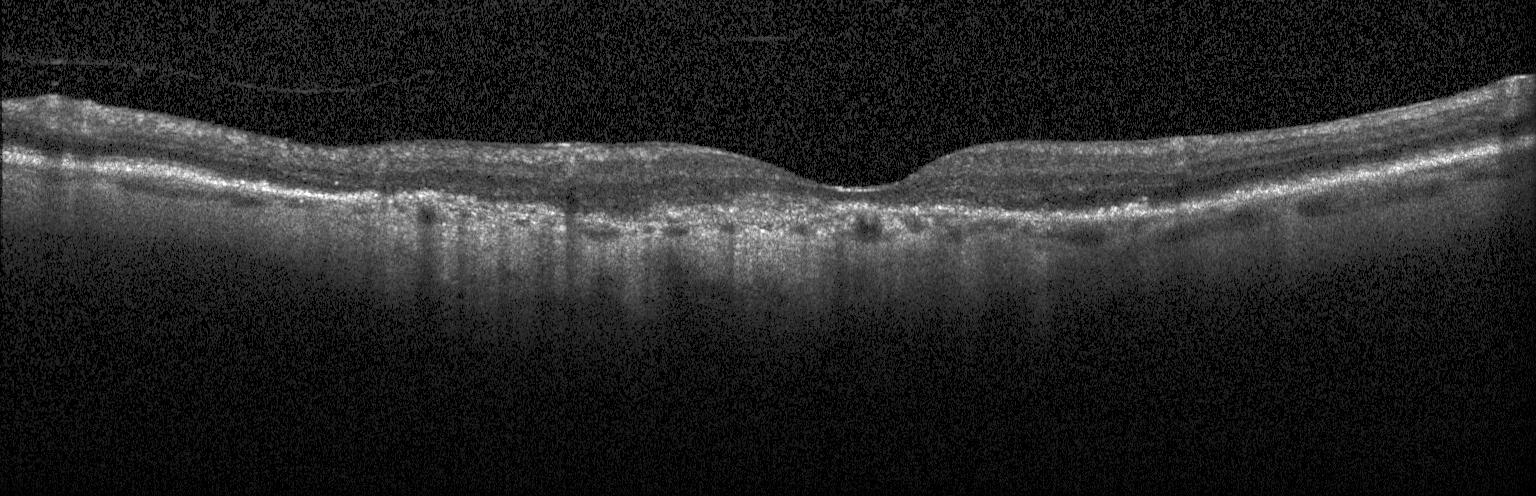
OCT finding: choroidal neovascularization.